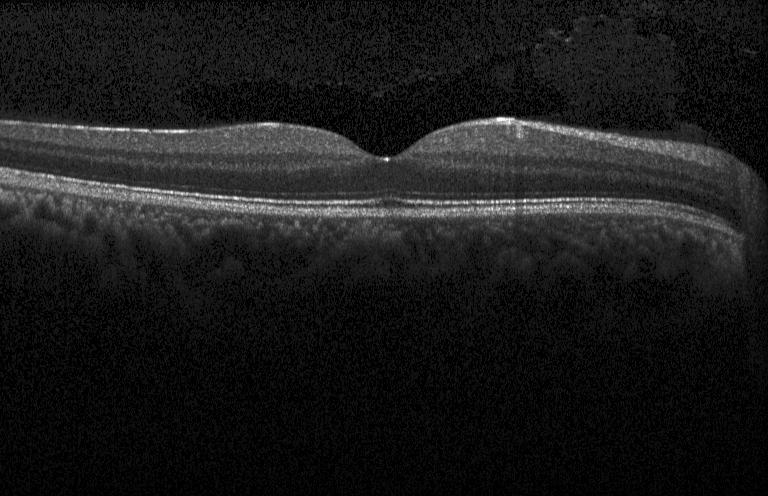 Finding: no evidence of CNV, DME, or drusen.